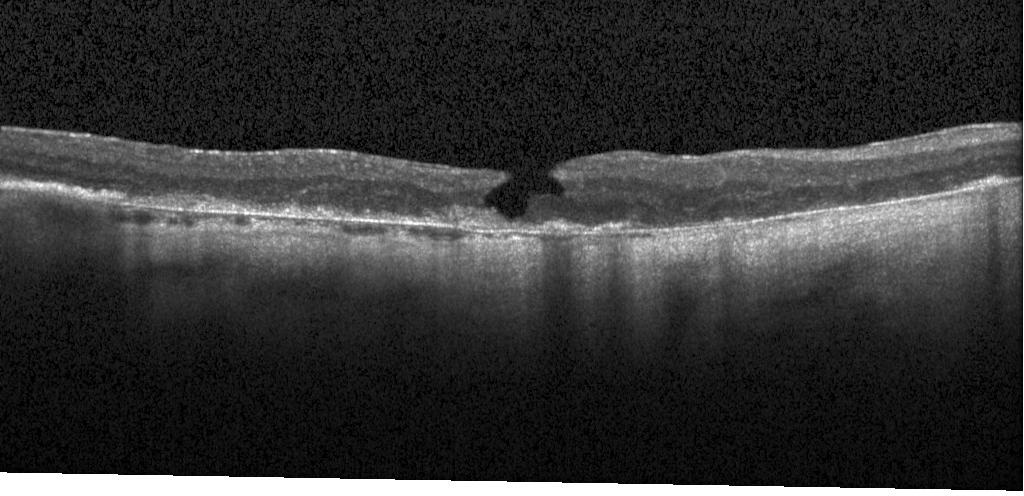 Dx: a choroidal neovascular membrane.